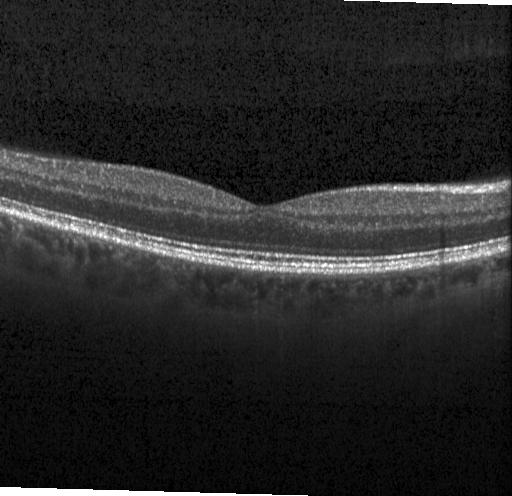

Retinal OCT cross-section showing neither choroidal neovascularization, diabetic macular edema, nor drusen.